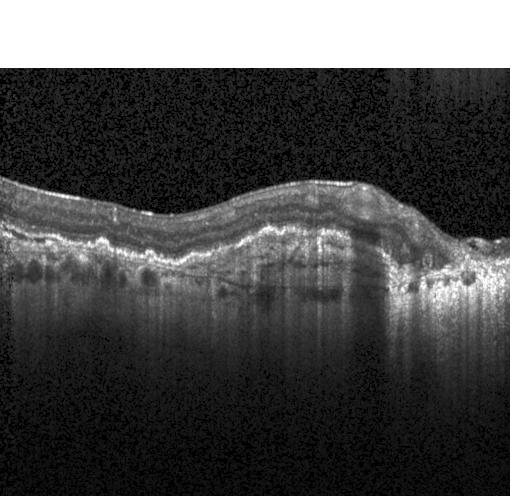

Heidelberg Spectralis OCT system, optical coherence tomography scan — Assessment: CNV.